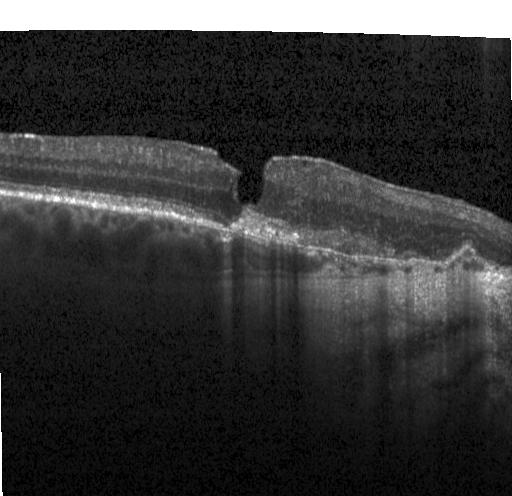

Spectral-domain OCT B-scan: CNV.